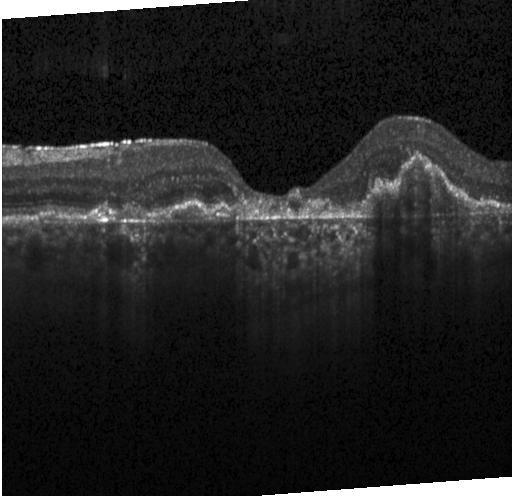 The scan shows a choroidal neovascular membrane.